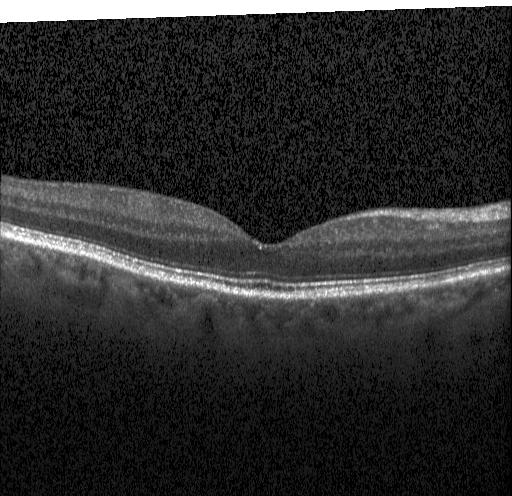
Optical coherence tomography scan; spectral-domain OCT; fovea-centered — Assessment: no choroidal neovascularization, no diabetic macular edema, and no drusen.